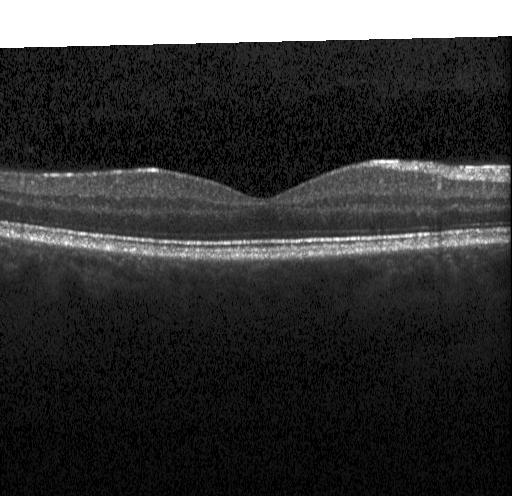 Diagnosis: no choroidal neovascularization, no diabetic macular edema, and no drusen.